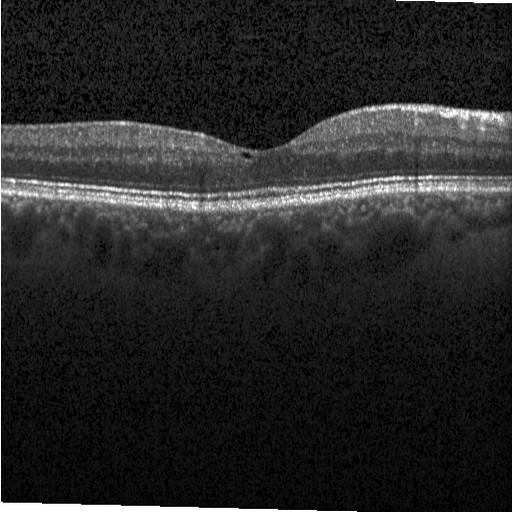 Acquired on a Heidelberg Spectralis, optical coherence tomography scan
This B-scan demonstrates diabetic macular edema.